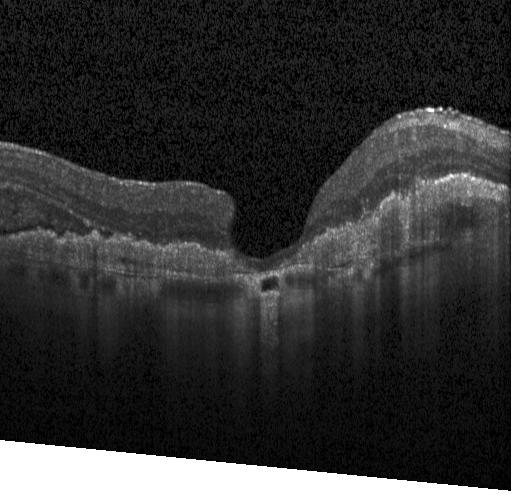

Diagnosis: a choroidal neovascular membrane.